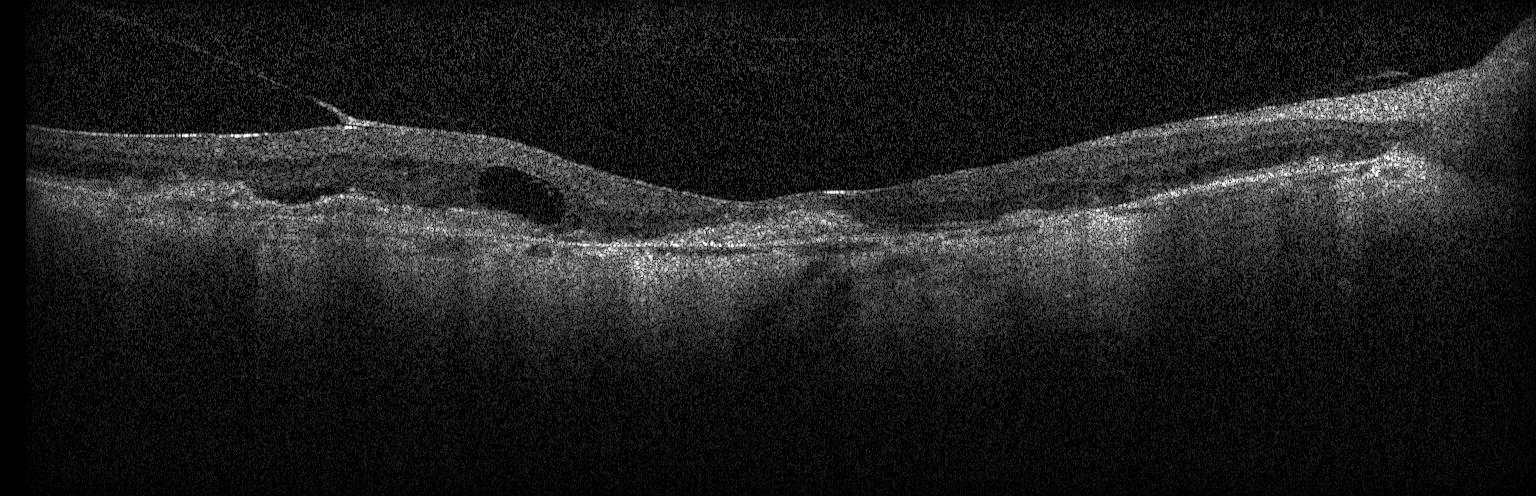

A choroidal neovascular membrane.